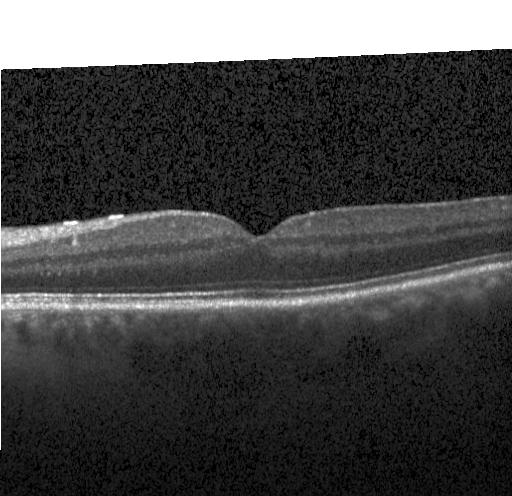 Macular OCT: no choroidal neovascularization, no diabetic macular edema, and no drusen.